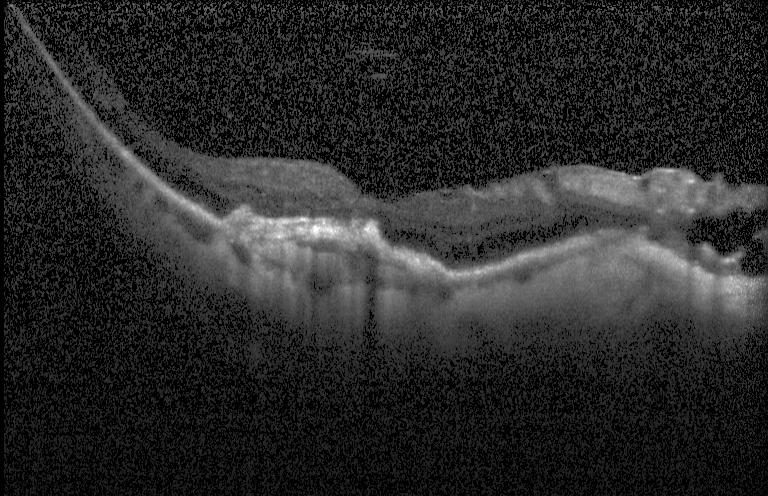 Macular OCT: CNV.